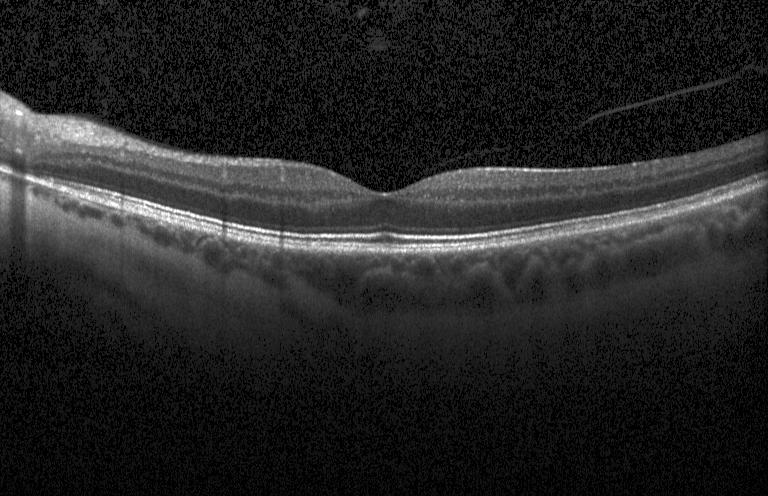

Optical coherence tomography scan — No CNV, DME, or drusen.